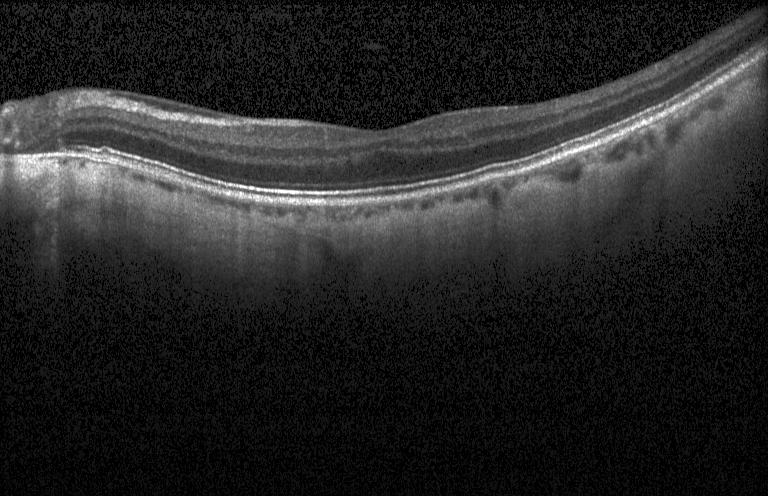

Macular OCT: neither choroidal neovascularization, diabetic macular edema, nor drusen.